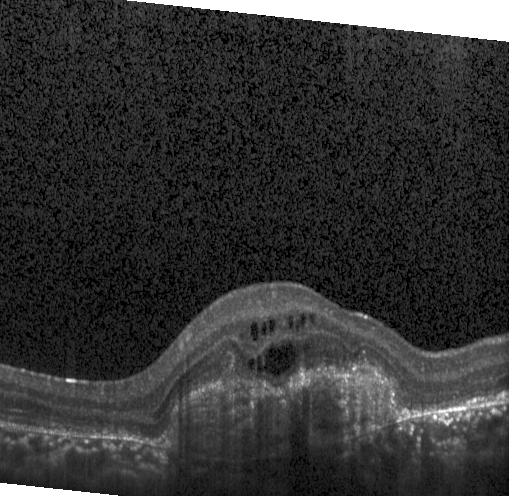 Fovea-centered · spectral-domain OCT · instrument: Heidelberg Spectralis · retinal OCT B-scan.
Diagnosis: a choroidal neovascular membrane.